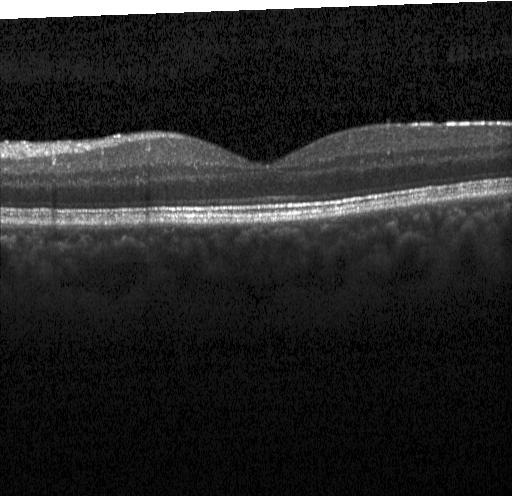 Retinal OCT cross-section showing no evidence of choroidal neovascularization, diabetic macular edema, or drusen.